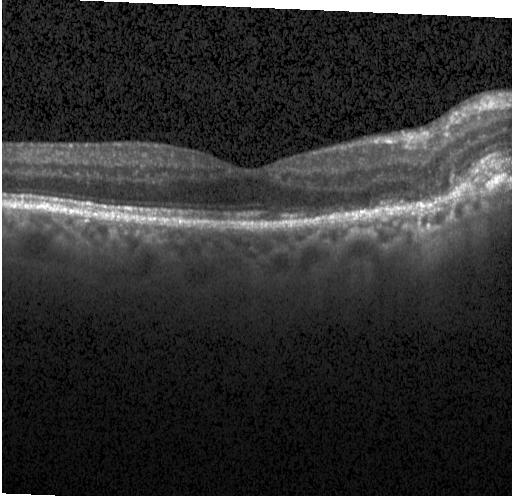
Optical coherence tomography B-scan; spectral-domain OCT; fovea-centered; Heidelberg Spectralis.
Impression: a choroidal neovascular membrane.